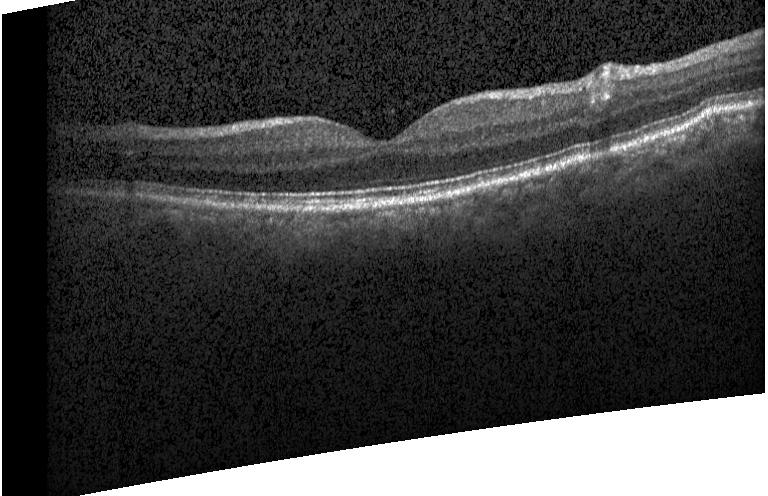 Retinal OCT B-scan; acquired on a Heidelberg Spectralis.
Finding: no choroidal neovascularization, diabetic macular edema, or drusen.